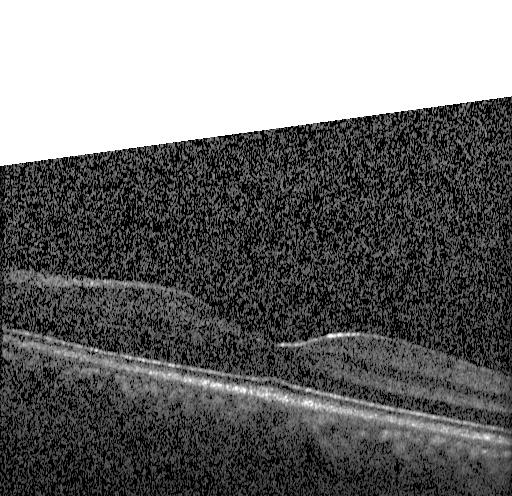 Dx: no evidence of CNV, DME, or drusen.